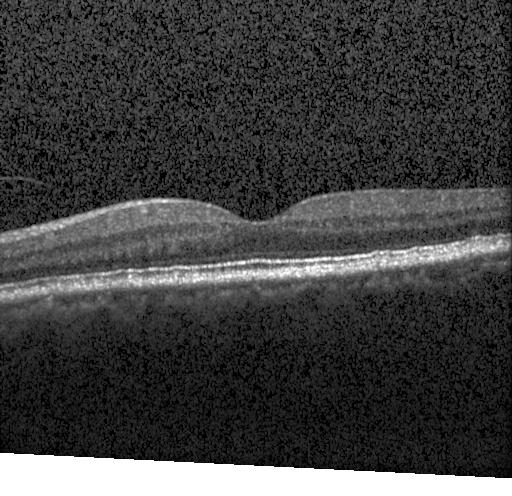
Diagnosis: no evidence of choroidal neovascularization, diabetic macular edema, or drusen.